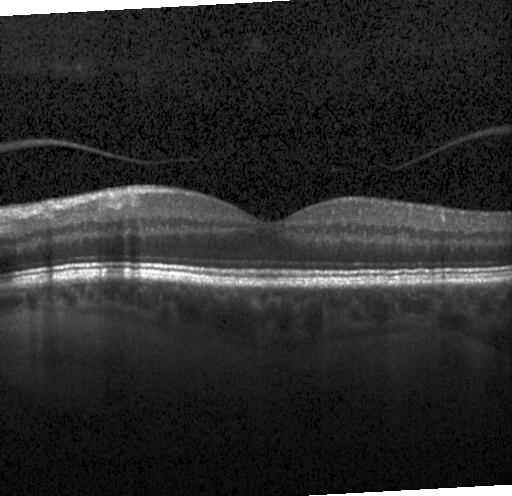

OCT scan showing neither CNV, DME, nor drusen.